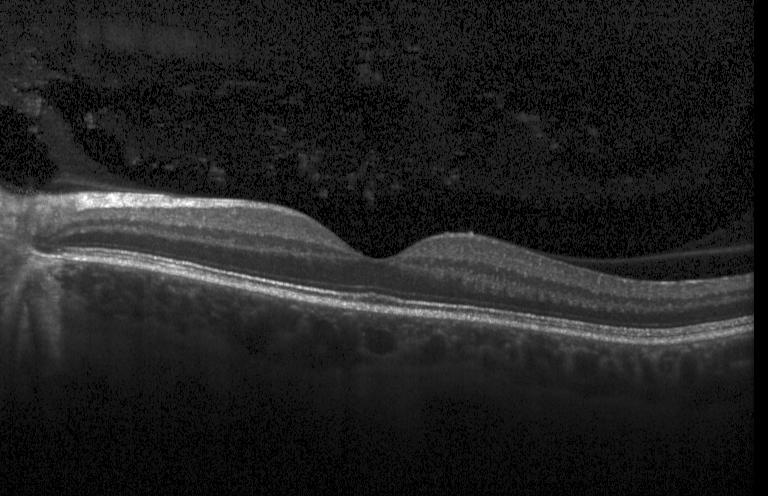
Spectral-domain OCT; retinal OCT cross-section; Heidelberg Spectralis
Impression: no CNV, no DME, and no drusen.